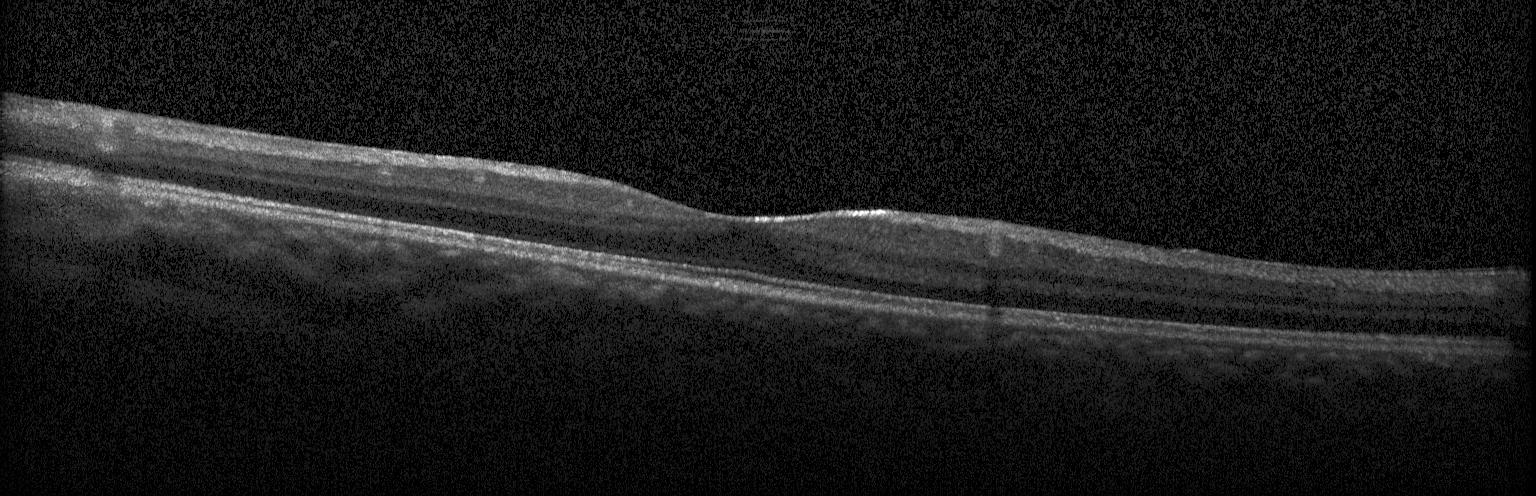
OCT B-scan
The scan shows neither CNV, DME, nor drusen.